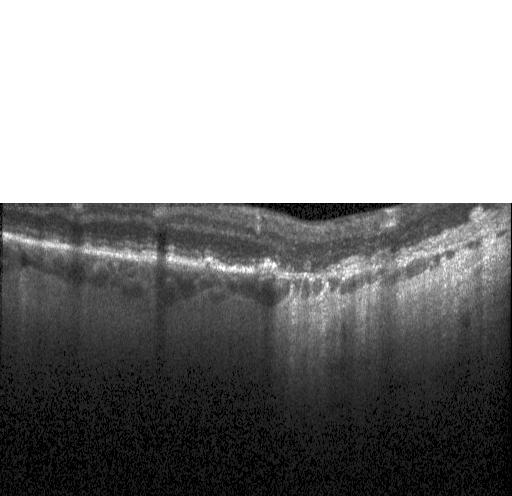

Finding: choroidal neovascularization (CNV).